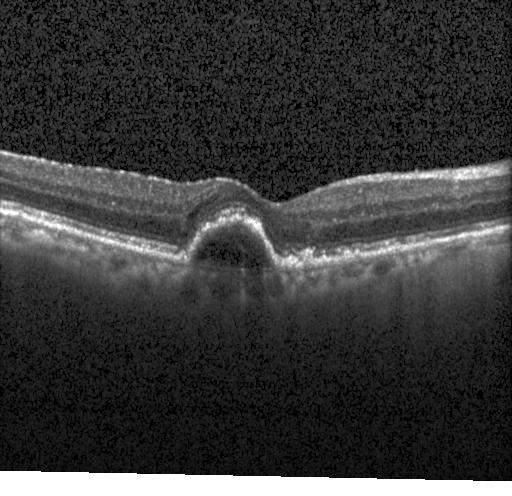 Heidelberg Spectralis, fovea-centered, OCT B-scan — Impression: CNV.